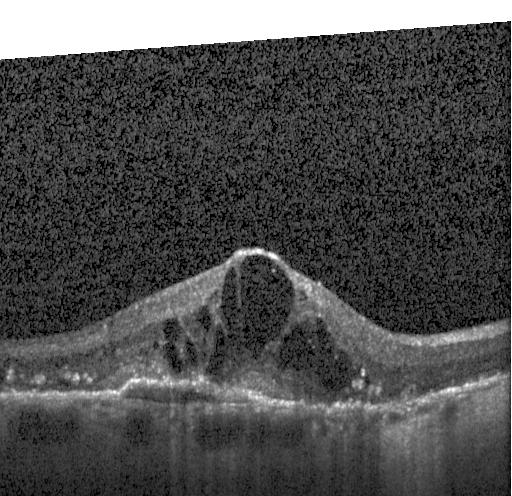 Optical coherence tomography scan. This B-scan demonstrates choroidal neovascularization.